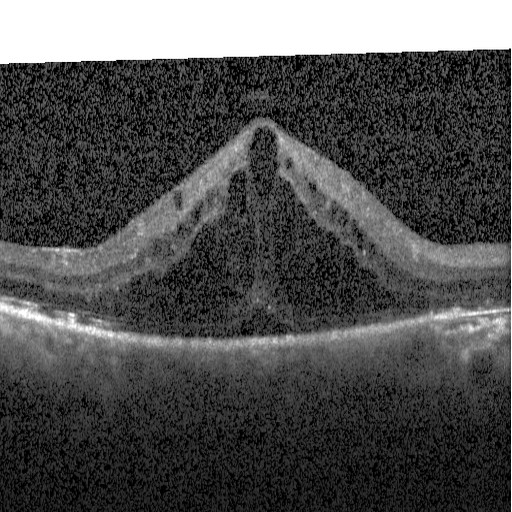
Spectral-domain OCT · Heidelberg Spectralis OCT system · retinal OCT B-scan · centered on the fovea.
Dx: diabetic macular edema (DME).